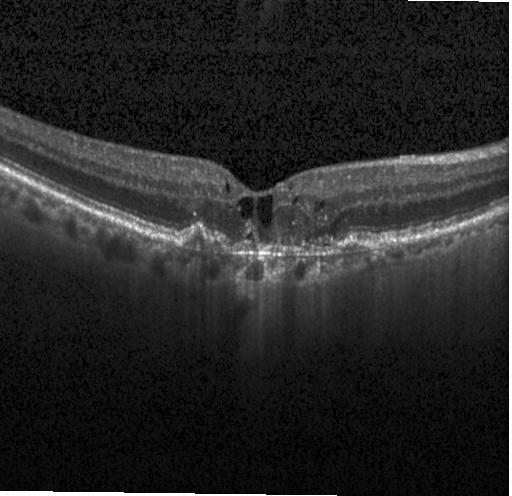
Retinal OCT B-scan
Assessment: a choroidal neovascular membrane.